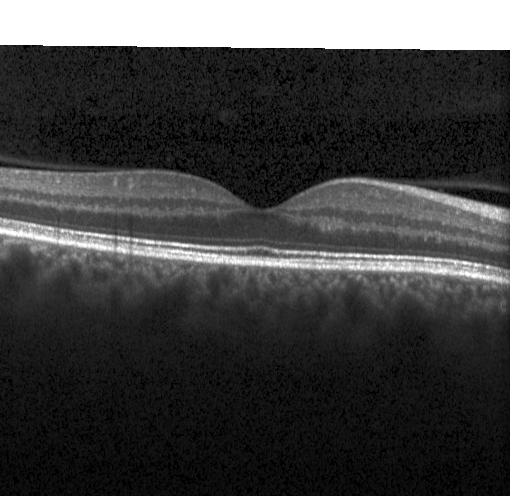
Spectral-domain OCT B-scan: no evidence of CNV, DME, or drusen.